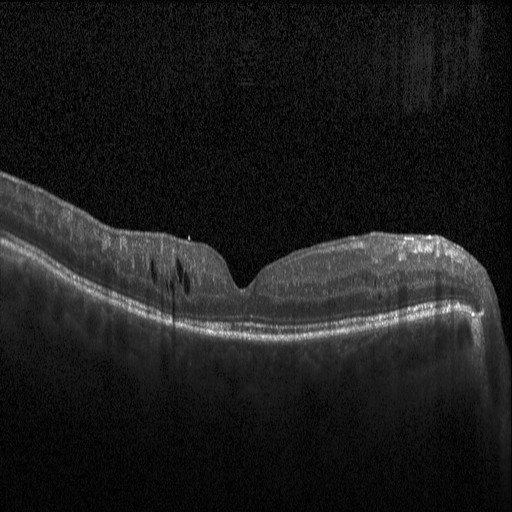

Diagnosis: diabetic macular edema (DME).